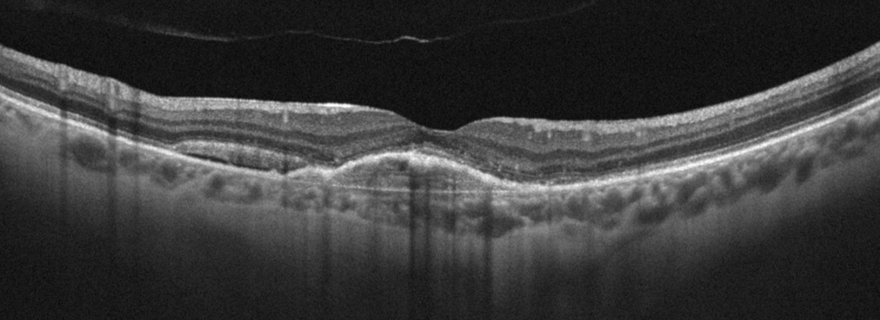

Dx: age-related macular degeneration.